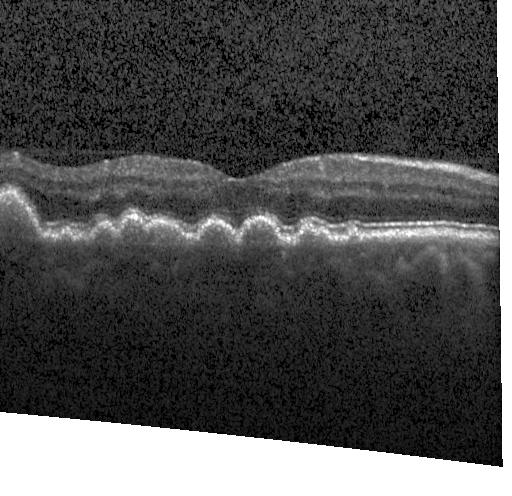

Heidelberg Spectralis; spectral-domain OCT; optical coherence tomography scan — Sub-RPE drusenoid deposits.